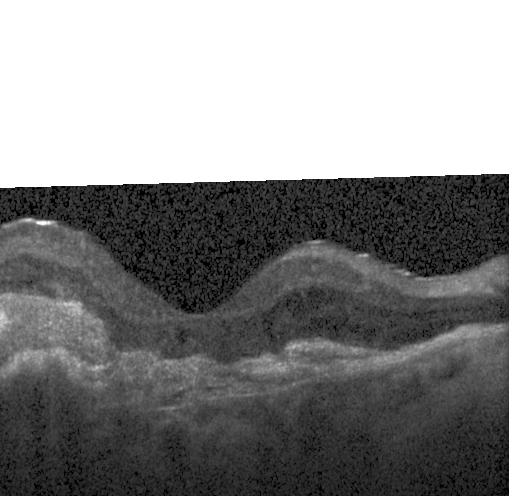

Fovea-centered · optical coherence tomography scan — Macular OCT: a choroidal neovascular membrane.